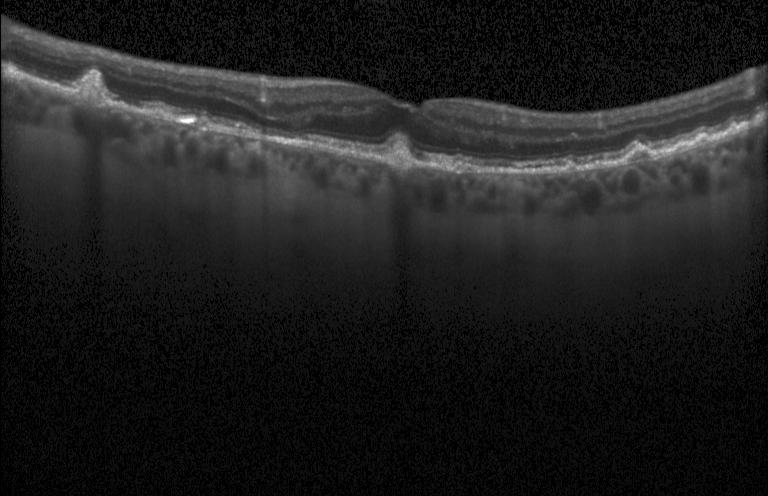 Instrument: Heidelberg Spectralis, retinal OCT B-scan, fovea-centered.
The scan shows multiple drusen.